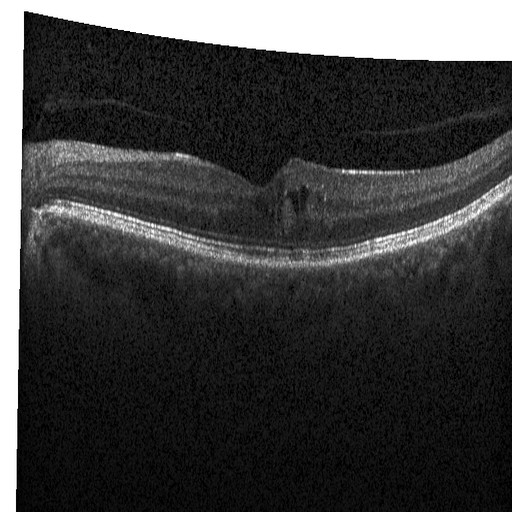

OCT B-scan · macular scan · Heidelberg Spectralis. Finding: diabetic macular edema.